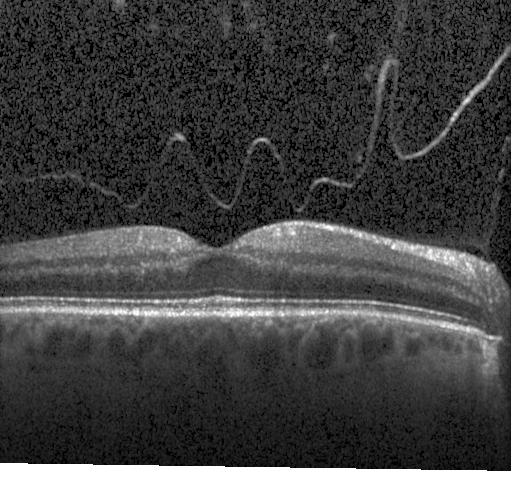 Through the macula. Spectral-domain optical coherence tomography. Heidelberg Spectralis. Optical coherence tomography scan.
This B-scan demonstrates no CNV, no DME, and no drusen.